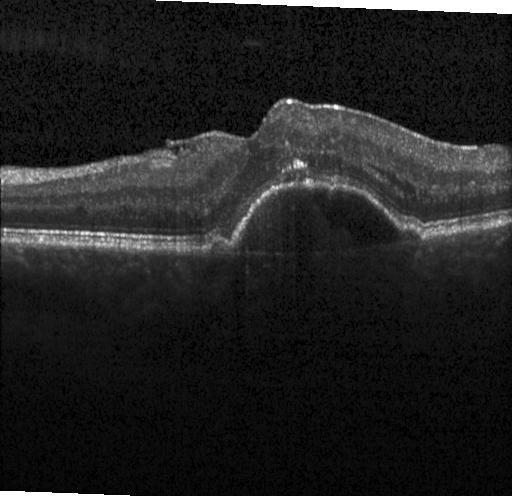
Diagnosis: choroidal neovascularization (CNV).